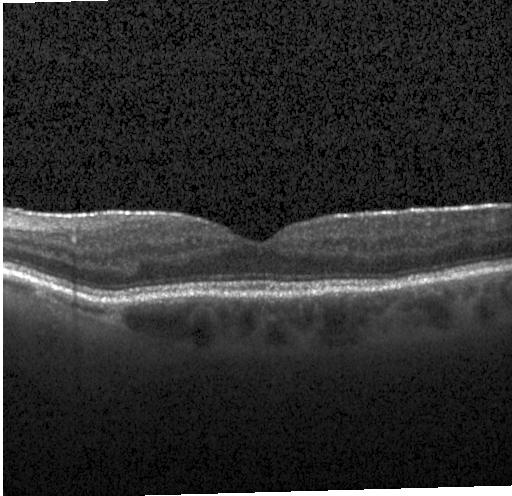 Macular OCT demonstrating neither choroidal neovascularization, diabetic macular edema, nor drusen.